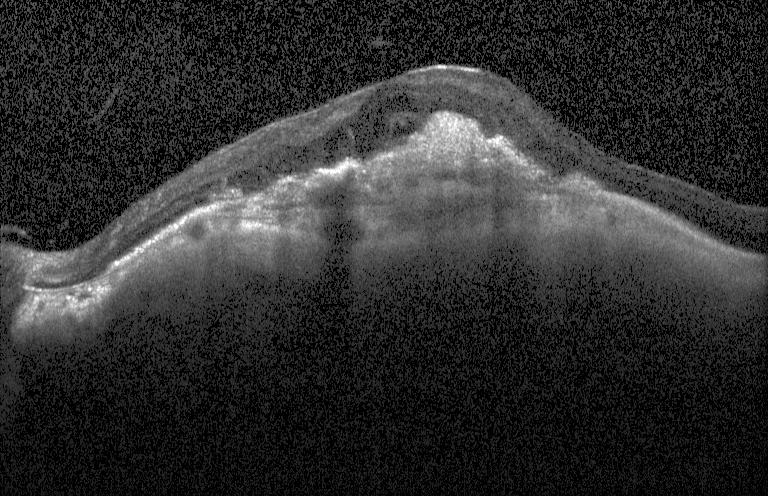
Impression: CNV.